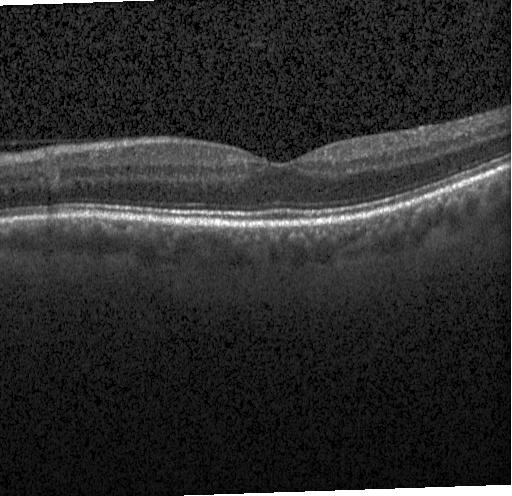

Spectral-domain OCT B-scan: no CNV, no DME, and no drusen.